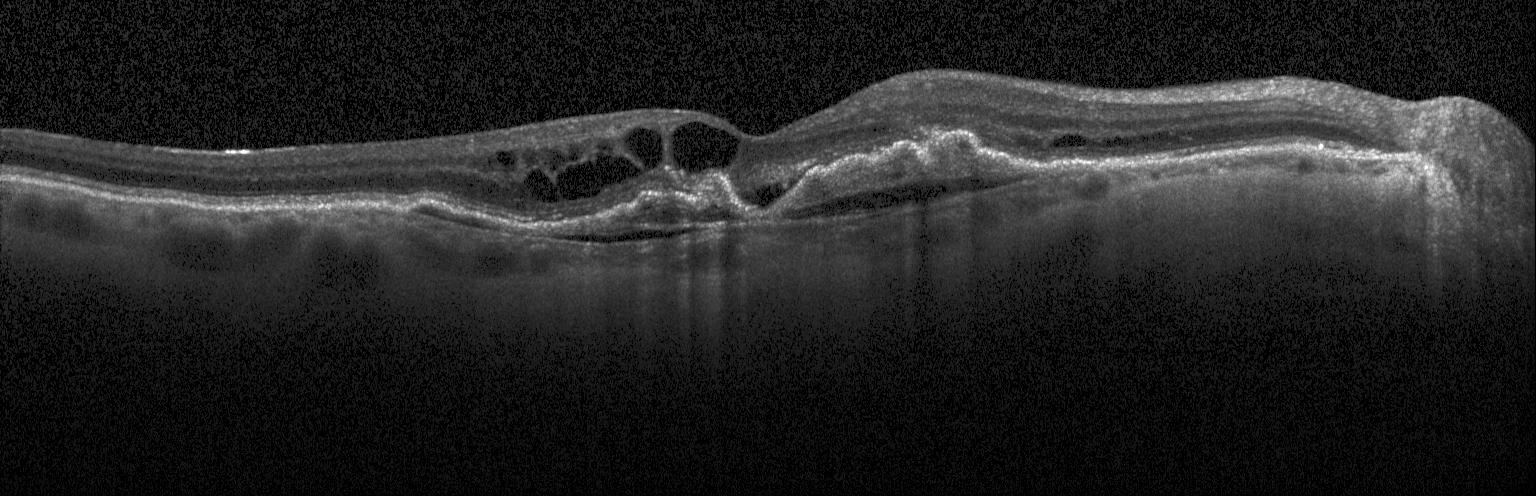 Fovea-centered, SD-OCT, optical coherence tomography B-scan — Impression: choroidal neovascularization (CNV).